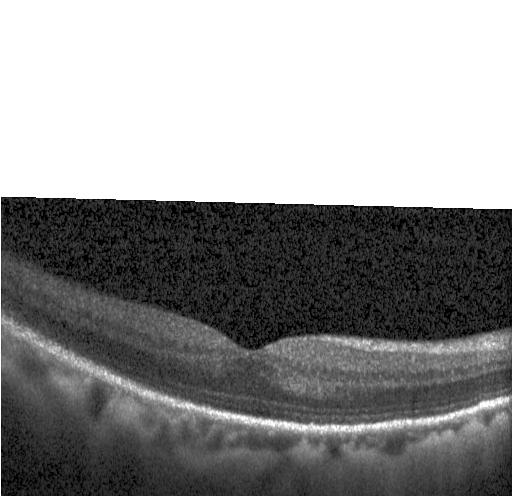
Optical coherence tomography B-scan — No evidence of choroidal neovascularization, diabetic macular edema, or drusen.